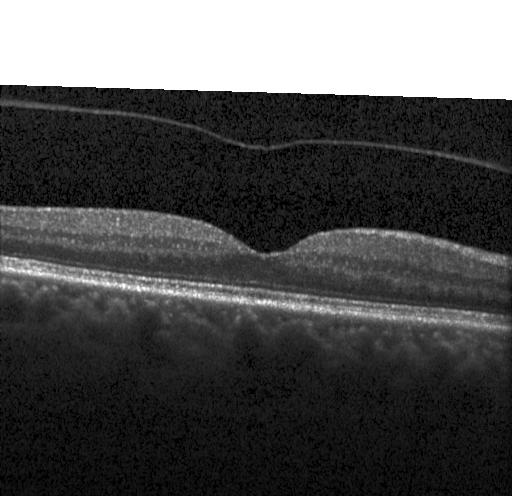

Optical coherence tomography scan. OCT finding: no evidence of CNV, DME, or drusen.